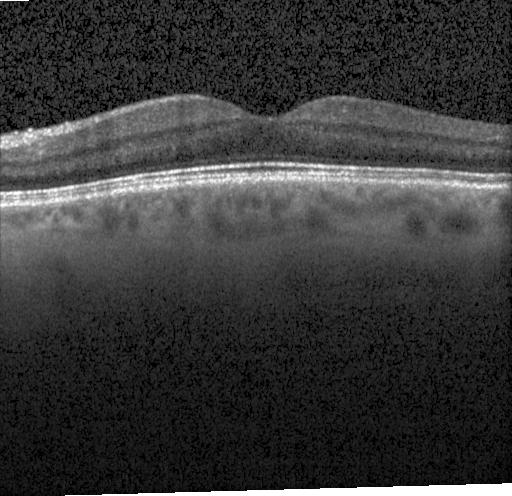
Diagnosis: no choroidal neovascularization, no diabetic macular edema, and no drusen.